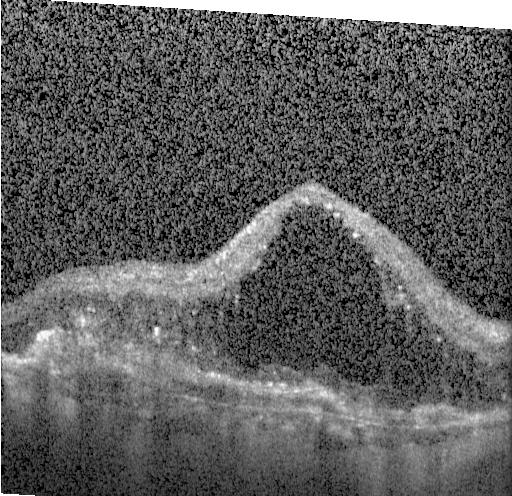 OCT B-scan · acquired on a Heidelberg Spectralis · spectral-domain optical coherence tomography. Diagnosis: choroidal neovascularization.